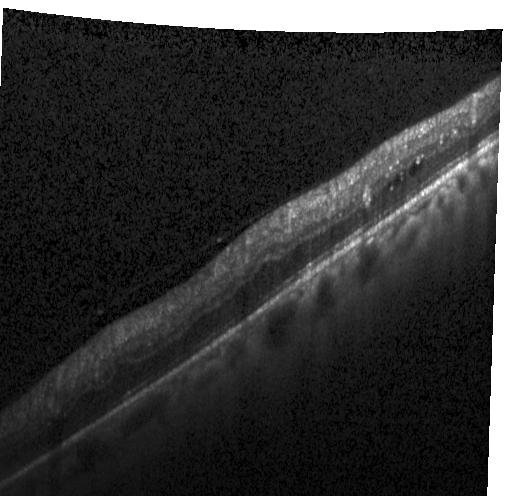

OCT scan showing diabetic macular edema (DME).